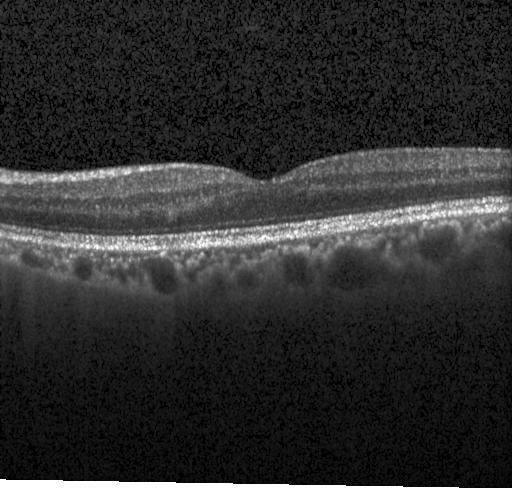
Spectral-domain OCT B-scan: neither CNV, DME, nor drusen.